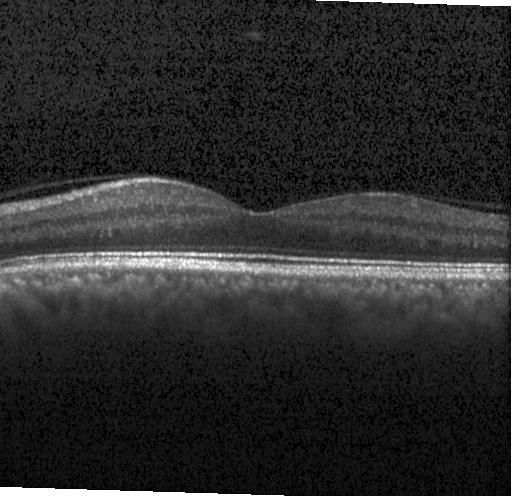

Retinal OCT B-scan · instrument: Heidelberg Spectralis · macular scan
OCT finding: no choroidal neovascularization, no diabetic macular edema, and no drusen.